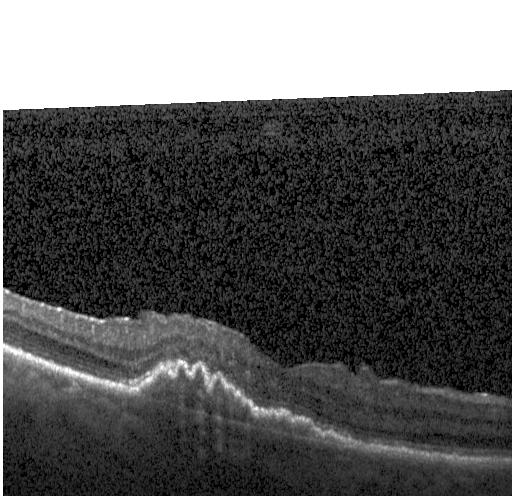 Retinal OCT cross-section. Acquired on a Heidelberg Spectralis. SD-OCT. Assessment: a choroidal neovascular membrane.